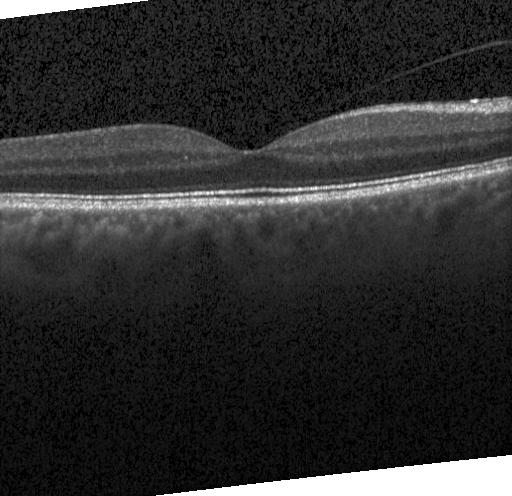 Centered on the fovea · optical coherence tomography B-scan — Diagnosis: no evidence of CNV, DME, or drusen.